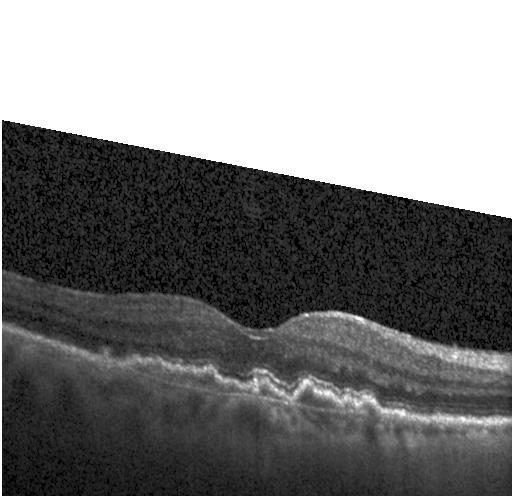
Retinal OCT B-scan
Macular OCT: a choroidal neovascular membrane.